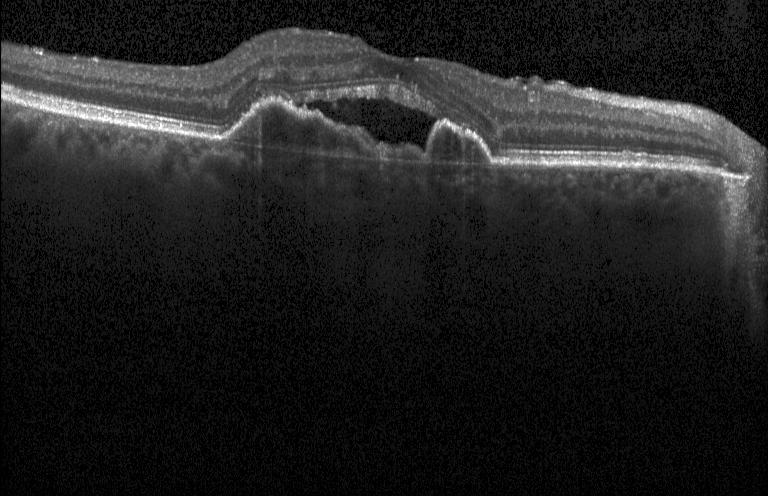
Horizontal scan through the fovea, acquired on a Heidelberg Spectralis, optical coherence tomography scan.
Impression: choroidal neovascularization (CNV).